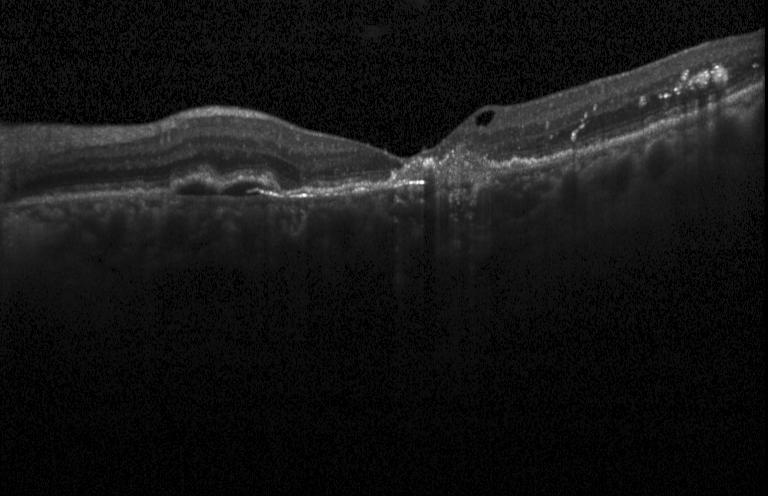 Spectral-domain optical coherence tomography. Heidelberg Spectralis. Optical coherence tomography scan.
Dx: a choroidal neovascular membrane.